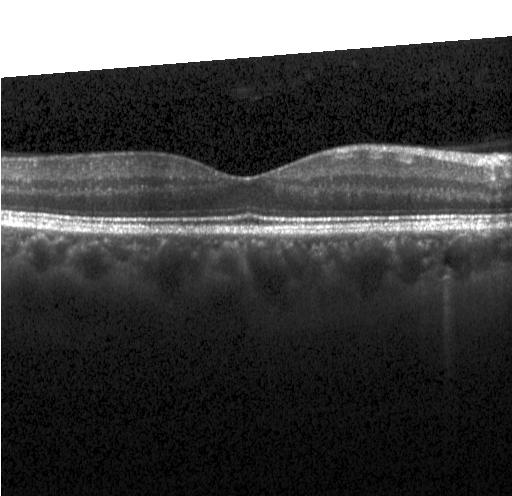

Impression: no choroidal neovascularization, diabetic macular edema, or drusen.